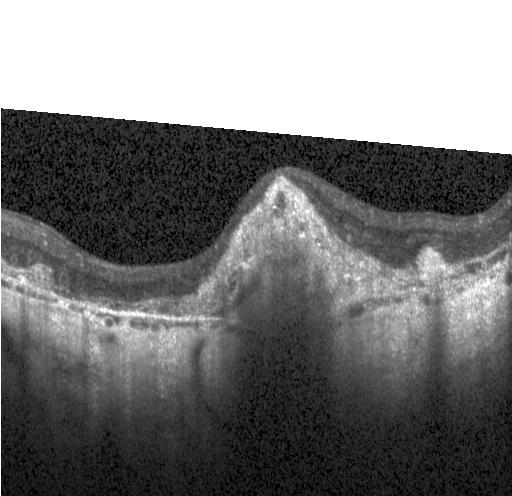
Spectral-domain optical coherence tomography · optical coherence tomography B-scan. Dx: a choroidal neovascular membrane.